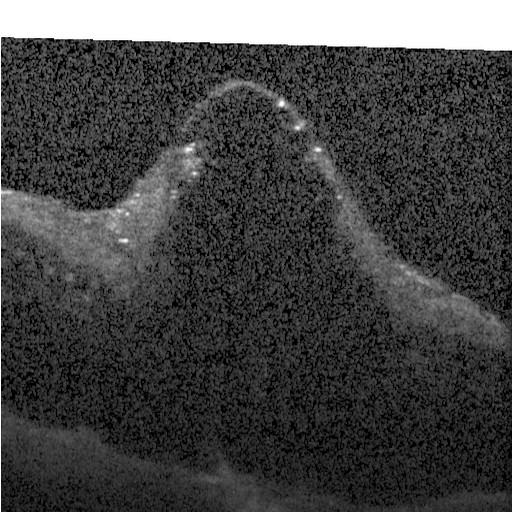

Optical coherence tomography B-scan. Diagnosis: diabetic macular edema (DME).